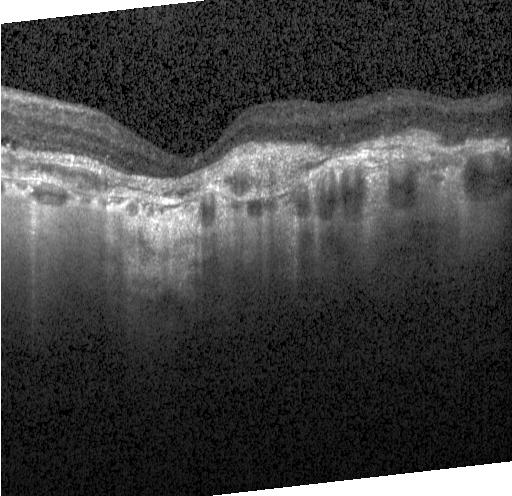 Heidelberg Spectralis. Horizontal scan through the fovea. SD-OCT. Optical coherence tomography B-scan. Impression: a choroidal neovascular membrane.